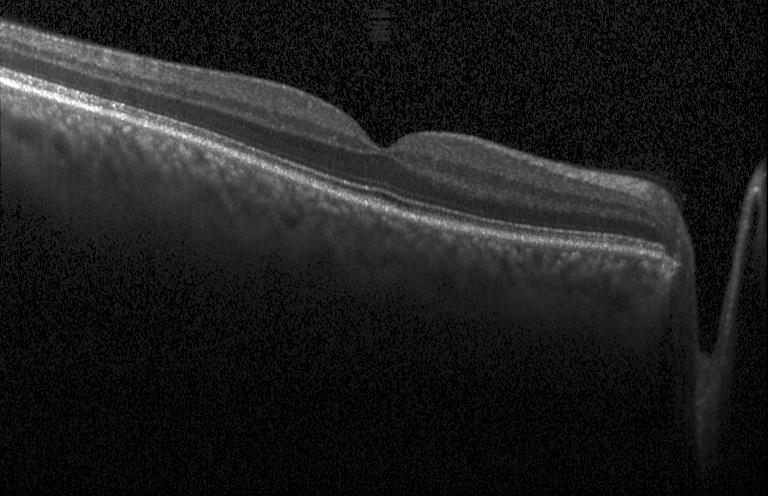
Dx: no choroidal neovascularization, diabetic macular edema, or drusen.